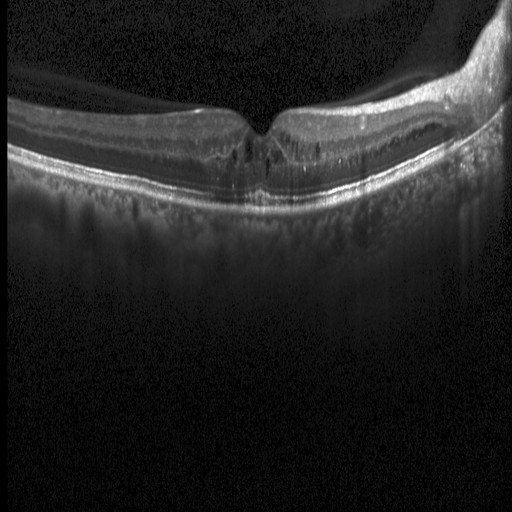
Retinal OCT cross-section showing diabetic macular edema.